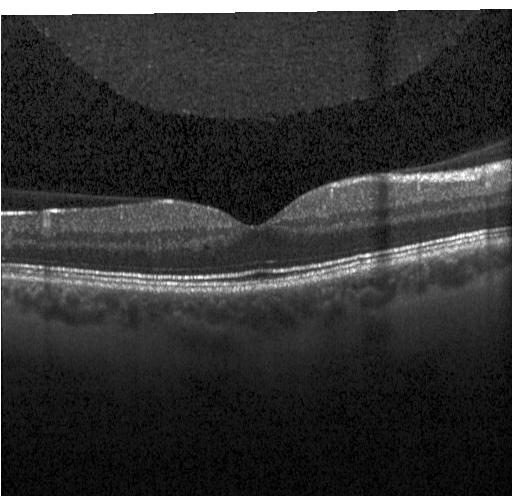
OCT B-scan, spectral-domain optical coherence tomography, Heidelberg Spectralis. Finding: neither choroidal neovascularization, diabetic macular edema, nor drusen.